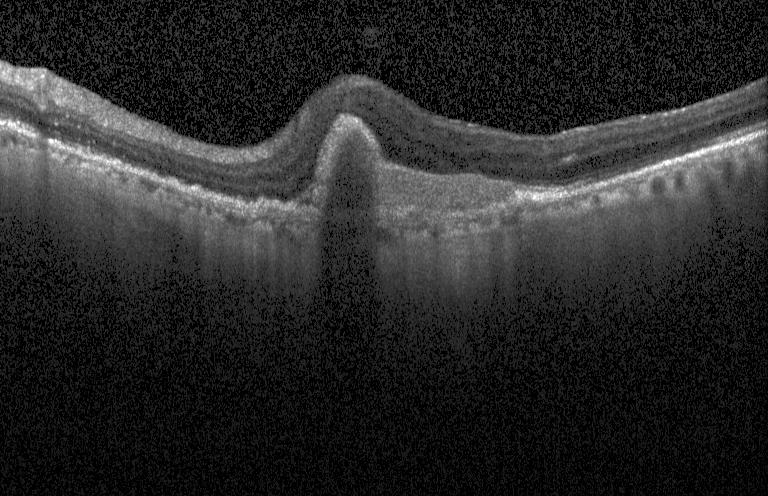 Optical coherence tomography scan, macular scan, instrument: Heidelberg Spectralis — Assessment: a choroidal neovascular membrane.